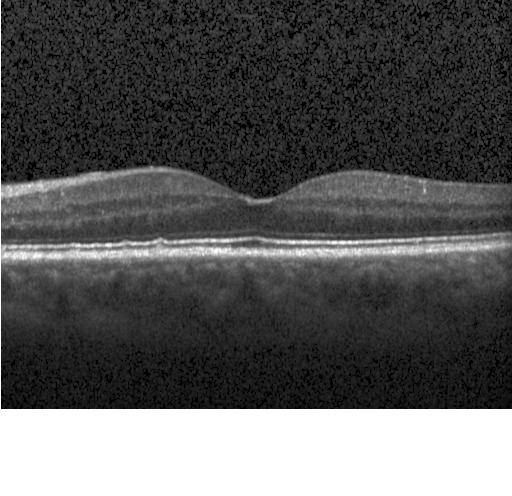 Spectral-domain OCT, OCT line scan.
Dx: sub-RPE drusenoid deposits.